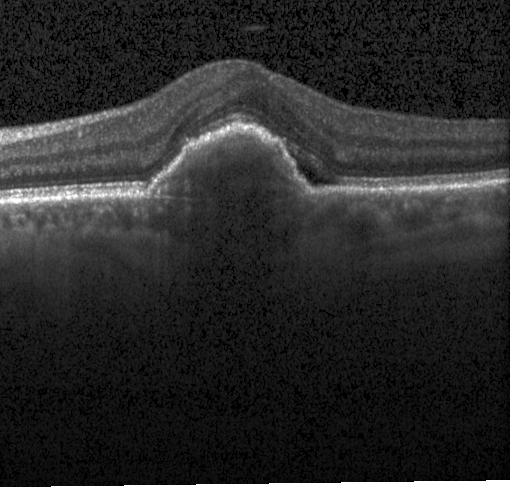
Fovea-centered; optical coherence tomography scan; spectral-domain optical coherence tomography; Heidelberg Spectralis.
Diagnosis: a choroidal neovascular membrane.